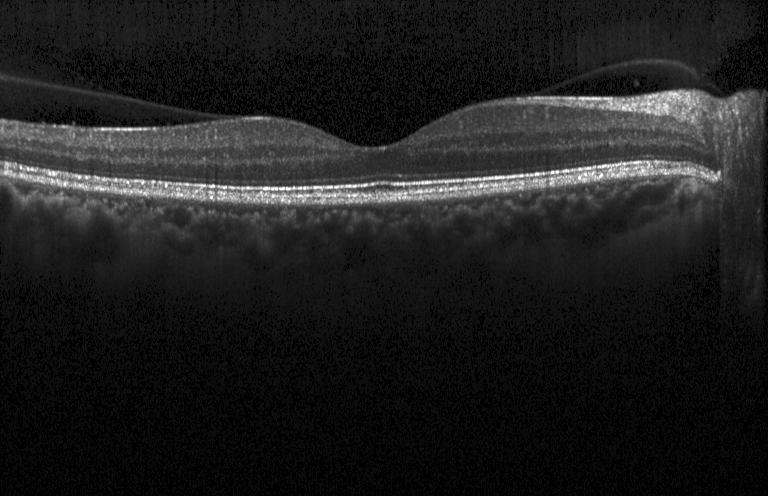

Retinal OCT cross-section, fovea-centered.
Diagnosis: neither CNV, DME, nor drusen.